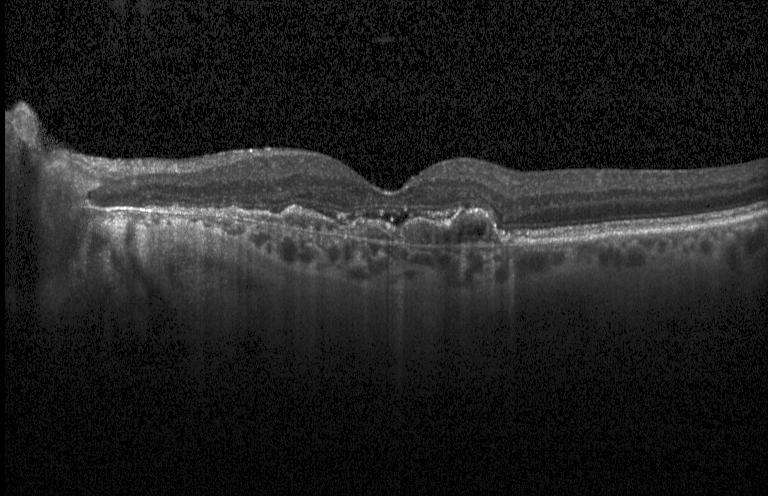

Dx: choroidal neovascularization.